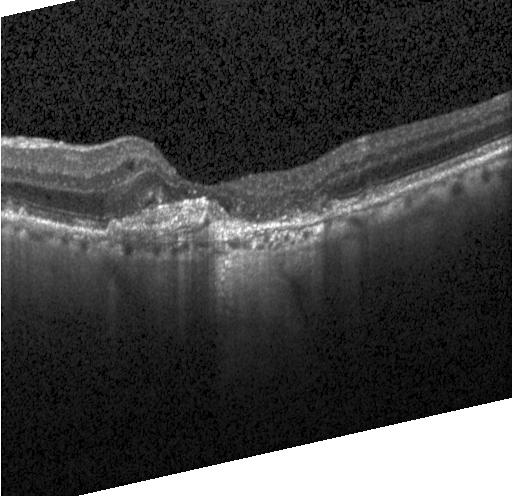 Retinal OCT B-scan. Heidelberg Spectralis. Spectral-domain OCT. Finding: a choroidal neovascular membrane.